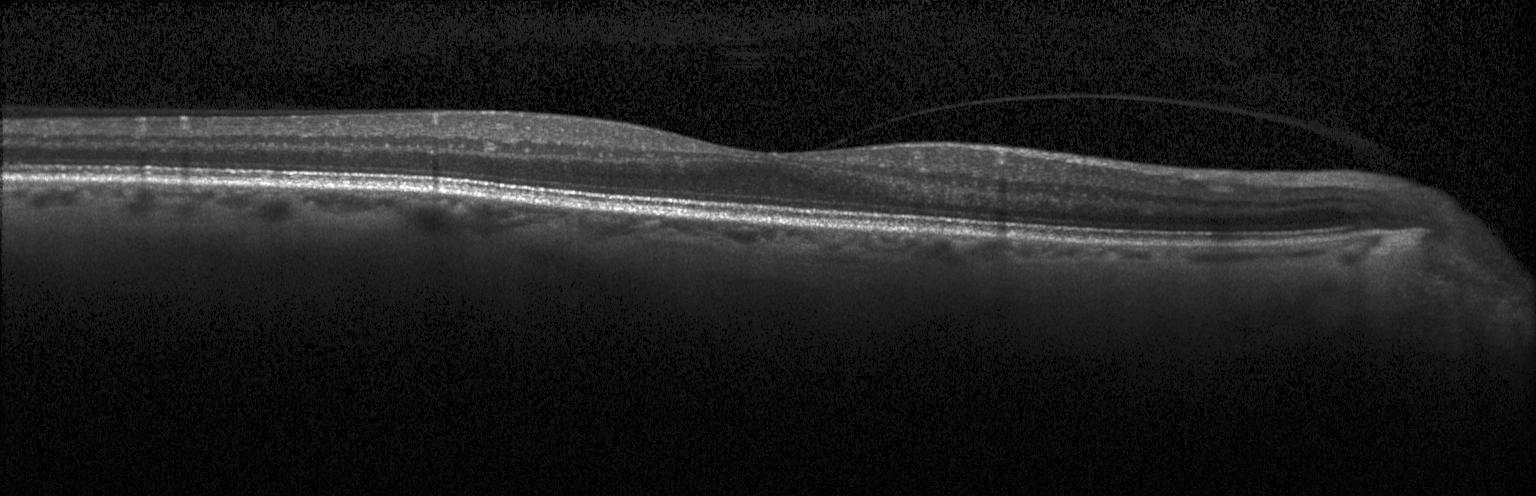 Dx: no choroidal neovascularization, no diabetic macular edema, and no drusen.